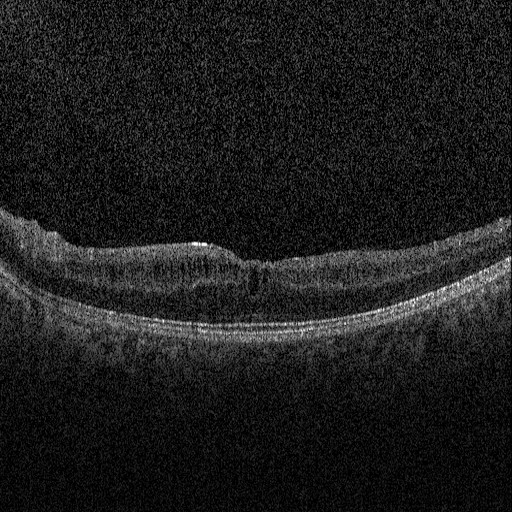

The scan shows diabetic macular edema.